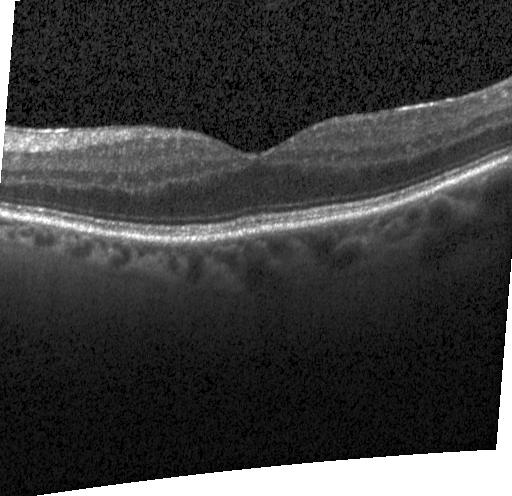
Optical coherence tomography scan. OCT finding: no evidence of CNV, DME, or drusen.